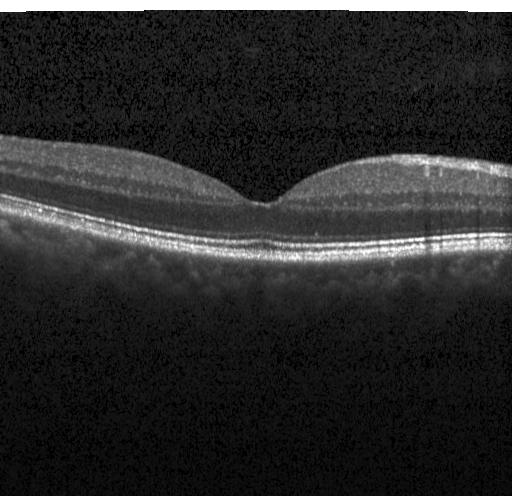
Instrument: Heidelberg Spectralis; optical coherence tomography B-scan; centered on the fovea
Diagnosis: no evidence of CNV, DME, or drusen.